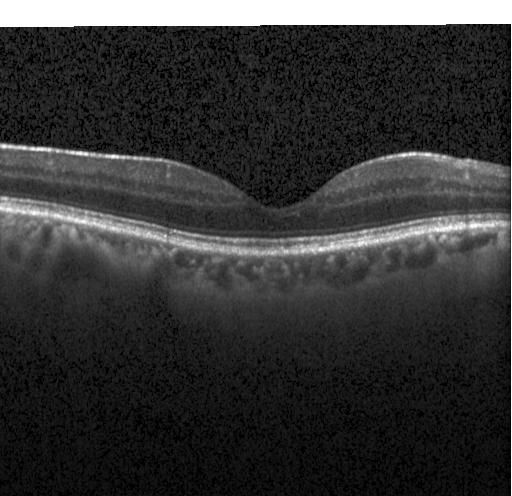
Through the macula; SD-OCT; OCT line scan; instrument: Heidelberg Spectralis. Assessment: no choroidal neovascularization, no diabetic macular edema, and no drusen.